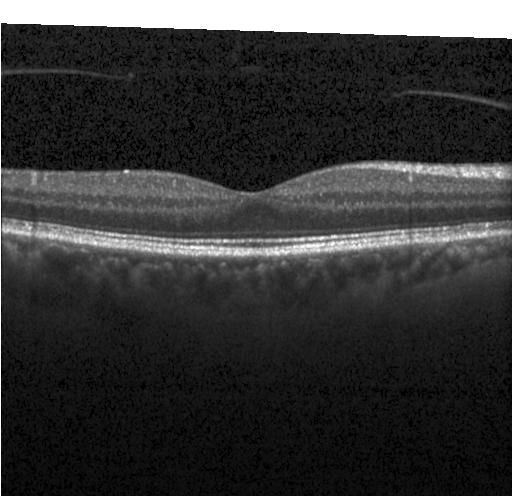
Retinal OCT cross-section · macular scan · Heidelberg Spectralis. Finding: neither choroidal neovascularization, diabetic macular edema, nor drusen.